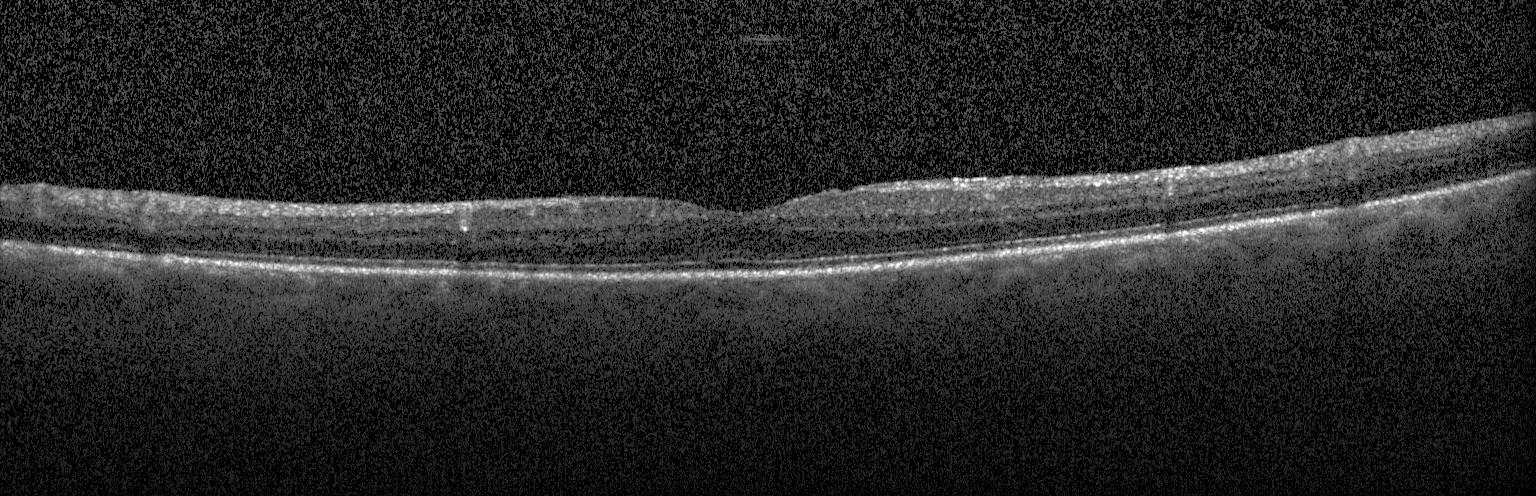

Retinal OCT B-scan. Impression: no CNV, no DME, and no drusen.